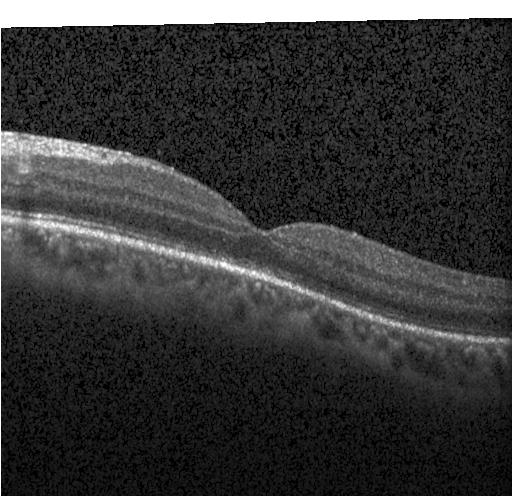

Impression: no CNV, DME, or drusen.